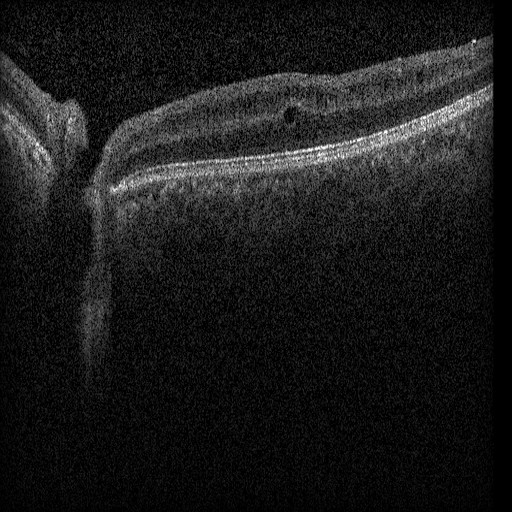

Fovea-centered; optical coherence tomography scan; Heidelberg Spectralis OCT system; spectral-domain OCT.
Diagnosis: diabetic macular edema (DME).